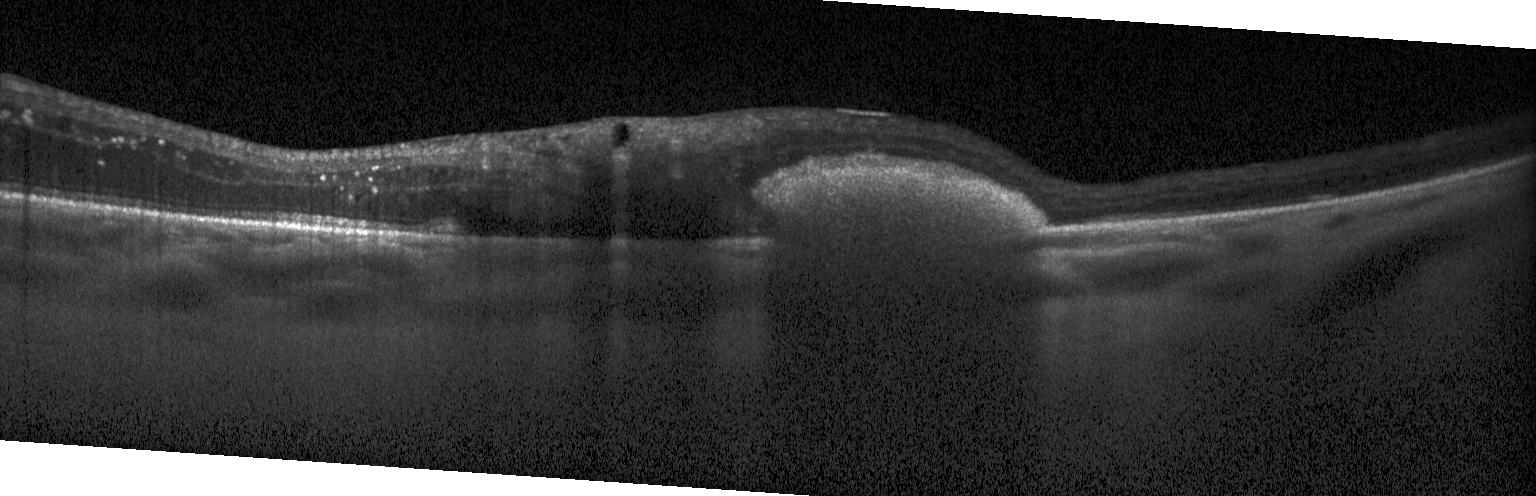 Macular OCT demonstrating CNV.